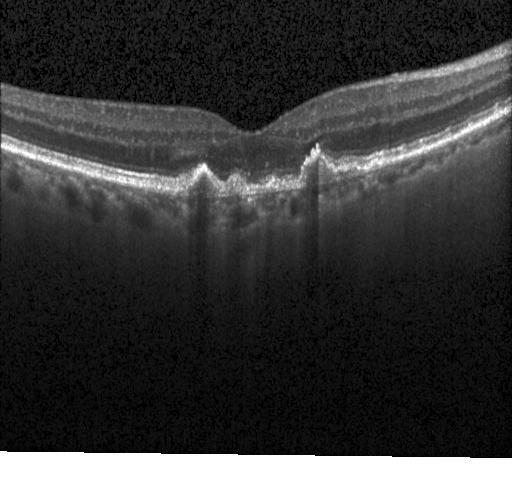
Spectral-domain optical coherence tomography · acquired on a Heidelberg Spectralis · retinal OCT cross-section.
Sub-RPE drusenoid deposits.